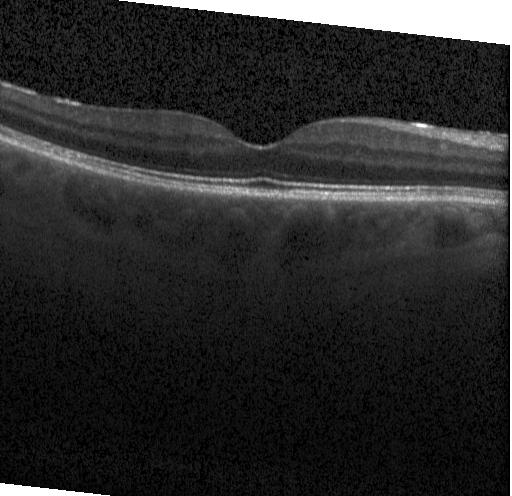 Diagnosis: no choroidal neovascularization, no diabetic macular edema, and no drusen.